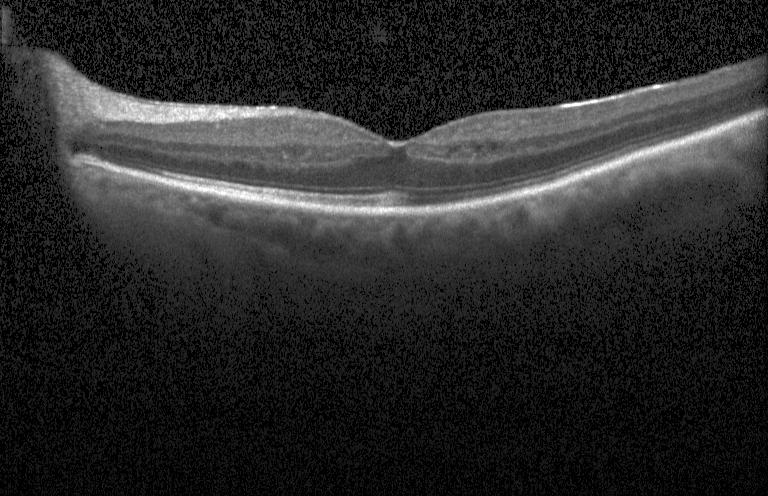 Diabetic macular edema.